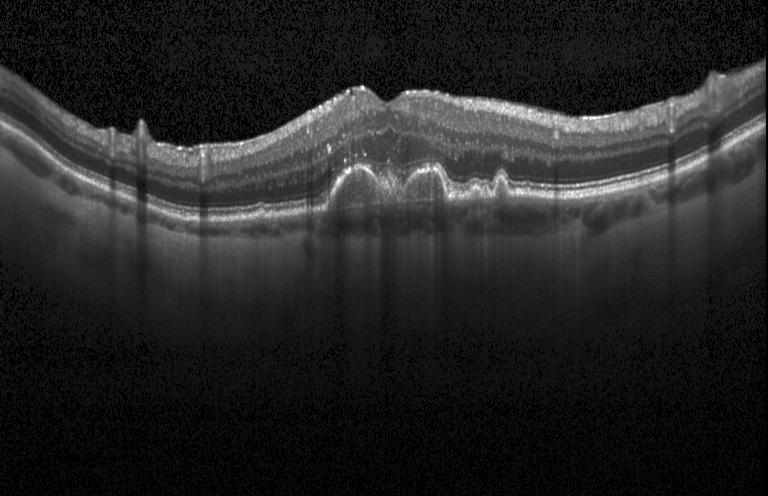 Dx: drusen.